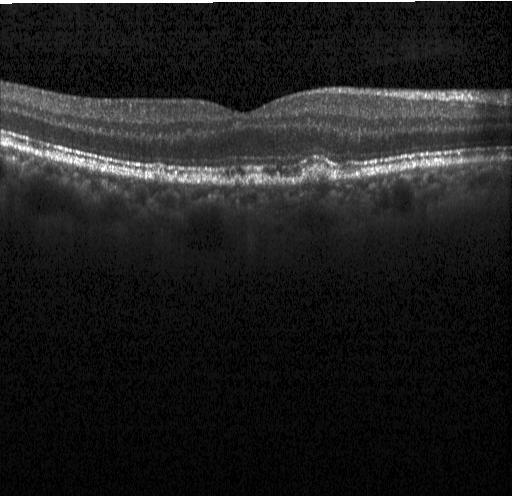
Retinal OCT cross-section showing sub-RPE drusenoid deposits.